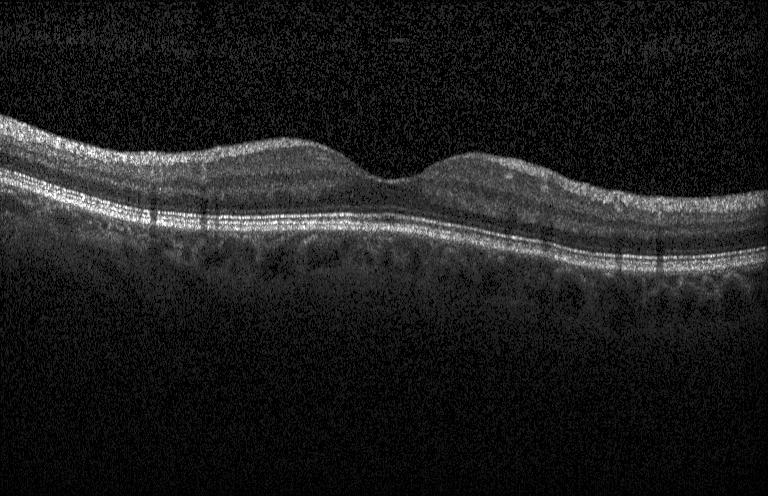
Optical coherence tomography scan — This B-scan demonstrates no evidence of CNV, DME, or drusen.